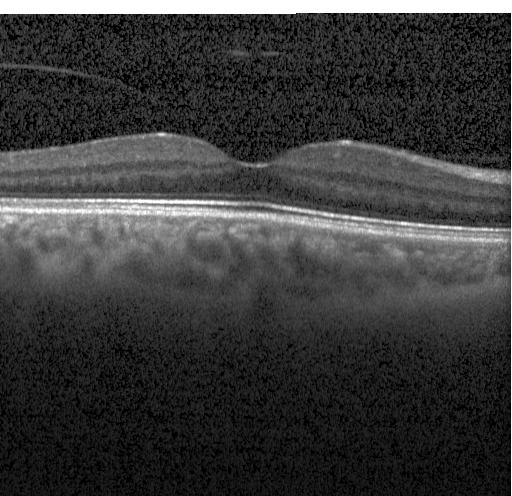
OCT B-scan showing neither choroidal neovascularization, diabetic macular edema, nor drusen.